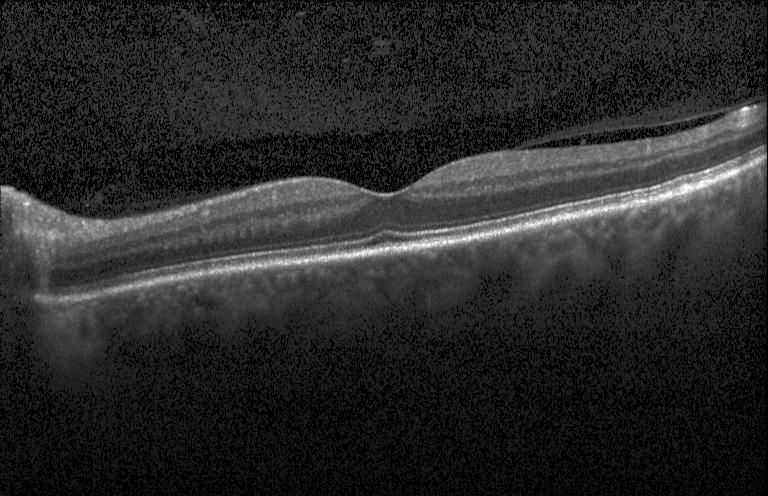

SD-OCT · acquired on a Heidelberg Spectralis · macular scan · OCT line scan — Impression: no evidence of choroidal neovascularization, diabetic macular edema, or drusen.